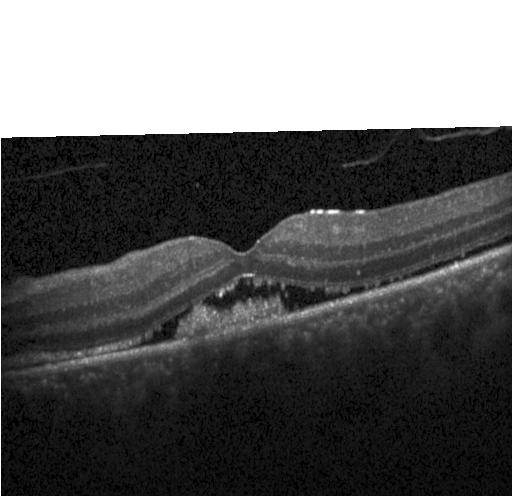 OCT scan showing a choroidal neovascular membrane.